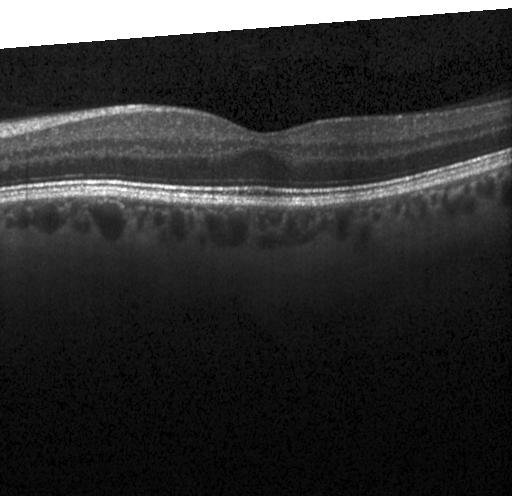

OCT line scan.
Finding: neither choroidal neovascularization, diabetic macular edema, nor drusen.